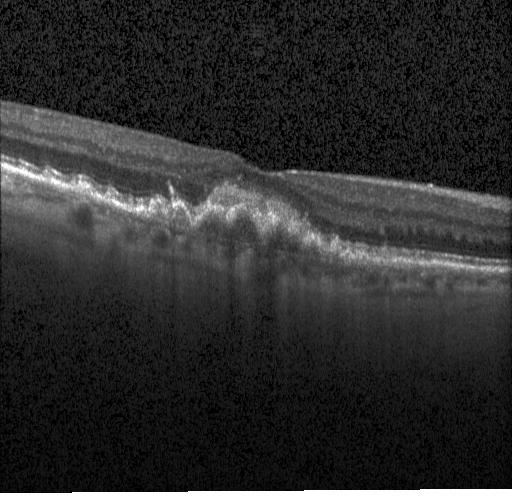
Spectral-domain optical coherence tomography · OCT line scan · acquired on a Heidelberg Spectralis · through the macula.
Choroidal neovascularization.